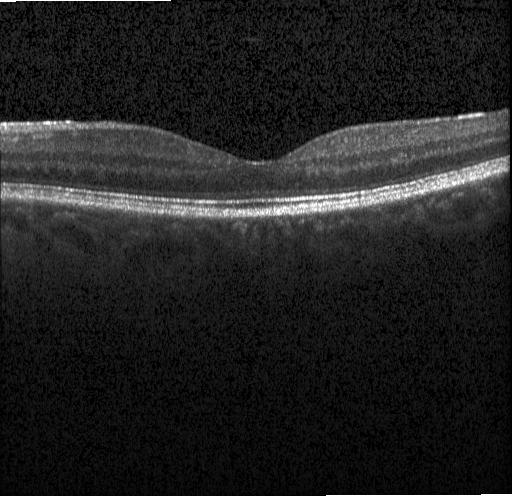 Finding: no CNV, no DME, and no drusen.